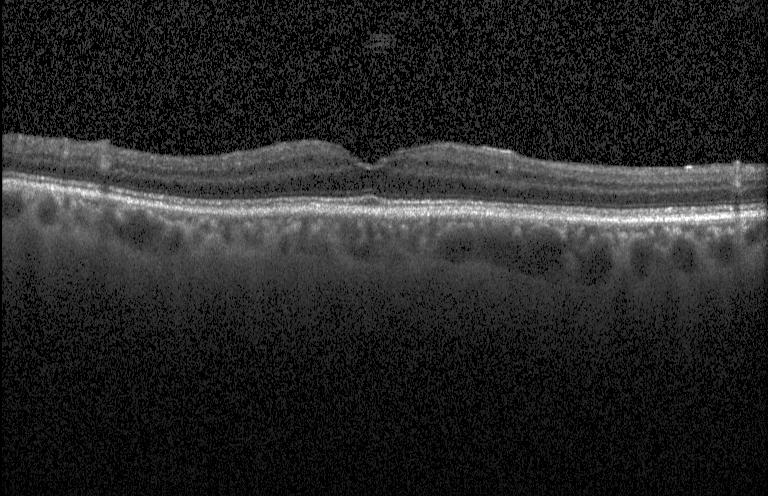 OCT line scan
Impression: neither choroidal neovascularization, diabetic macular edema, nor drusen.